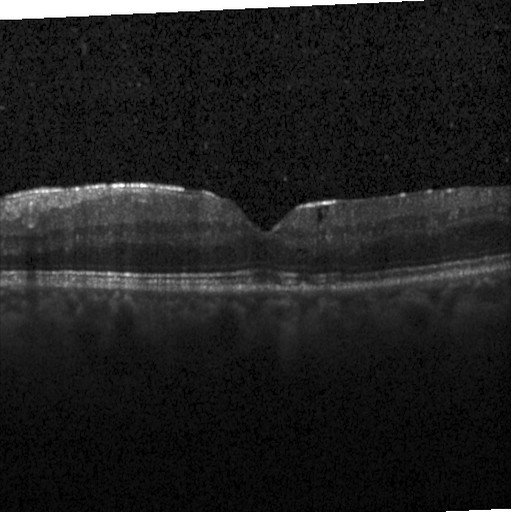 Heidelberg Spectralis, spectral-domain OCT, macular scan, OCT B-scan
Impression: diabetic macular edema (DME).